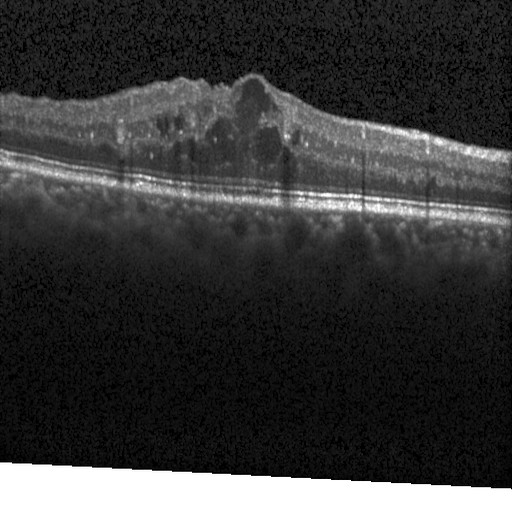
OCT B-scan
DME.